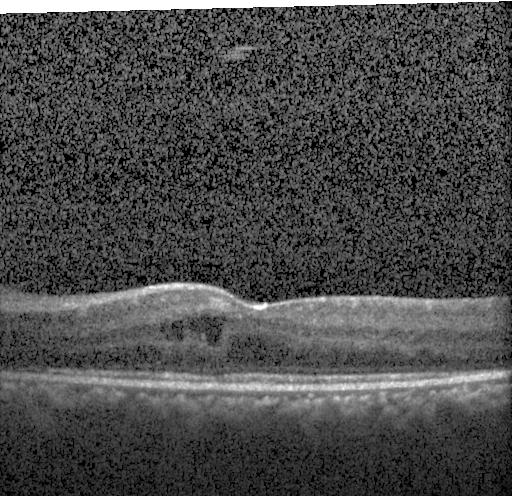
Horizontal scan through the fovea; spectral-domain OCT; OCT line scan
Diagnosis: DME.